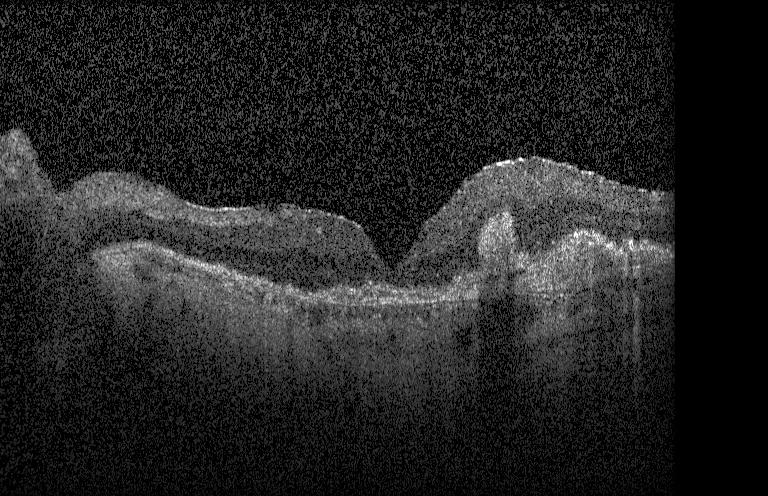 Impression: choroidal neovascularization (CNV).